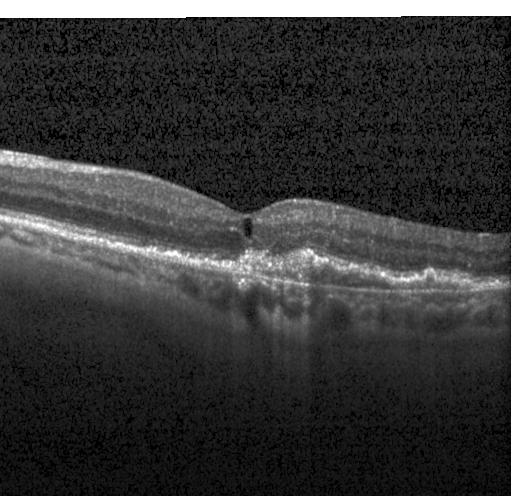

The scan shows a choroidal neovascular membrane.